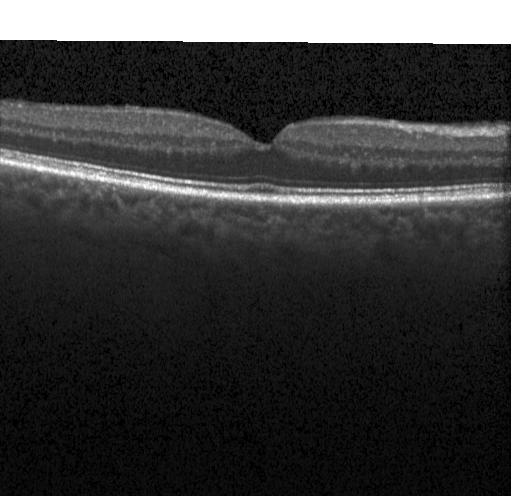
Impression: no evidence of CNV, DME, or drusen.